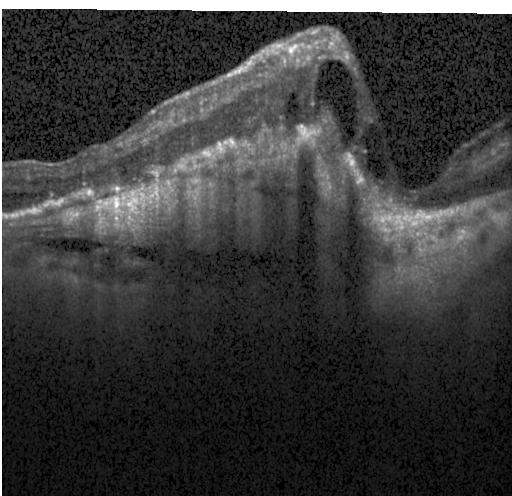 OCT line scan · instrument: Heidelberg Spectralis · centered on the fovea · spectral-domain OCT.
Impression: a choroidal neovascular membrane.